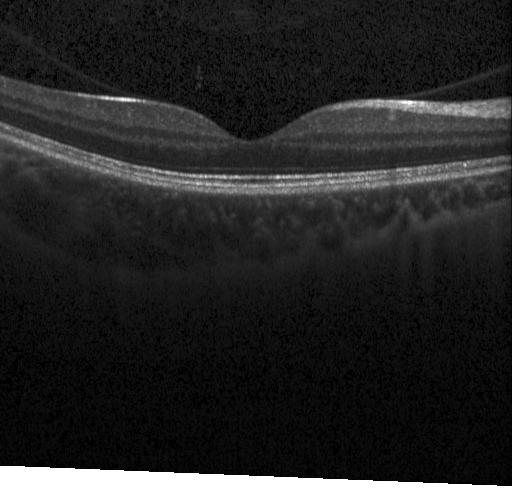

Through the macula, Heidelberg Spectralis, optical coherence tomography B-scan, spectral-domain OCT.
Assessment: no evidence of choroidal neovascularization, diabetic macular edema, or drusen.